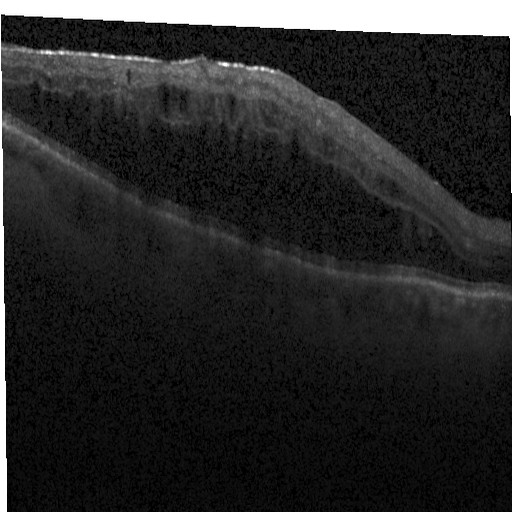 Retinal OCT B-scan — Diagnosis: DME.